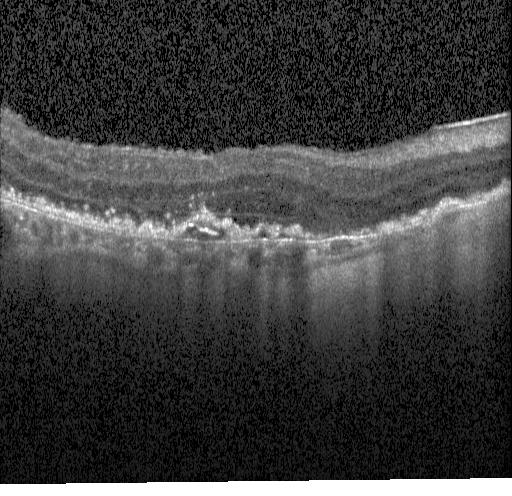 Finding: choroidal neovascularization (CNV).